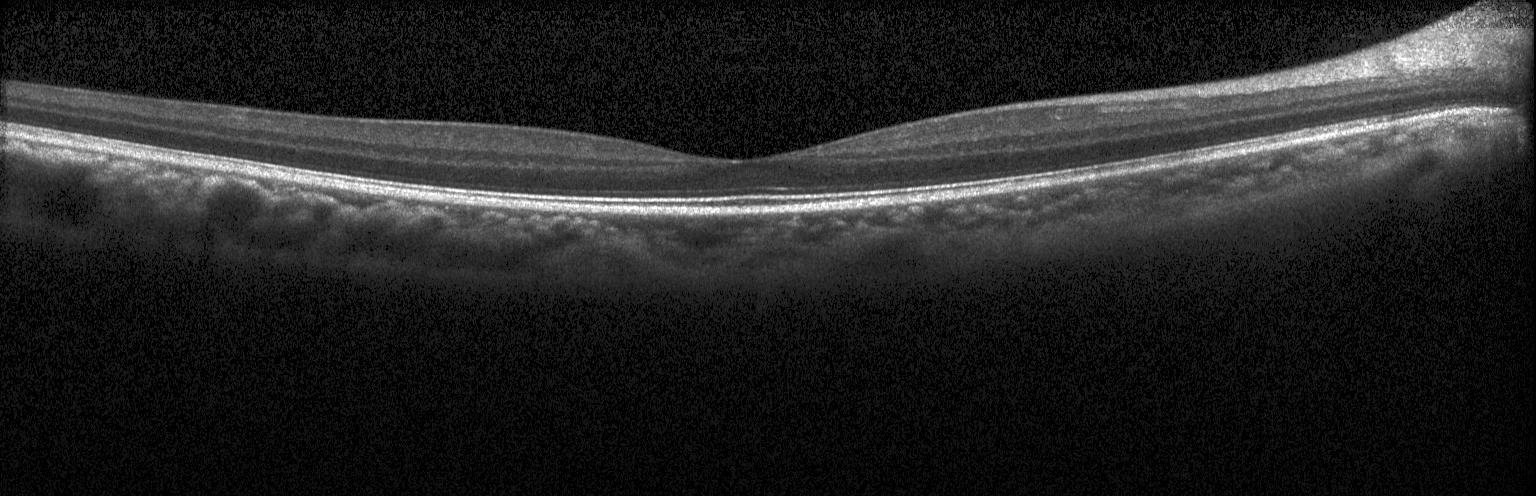

OCT B-scan, fovea-centered. Assessment: no CNV, no DME, and no drusen.